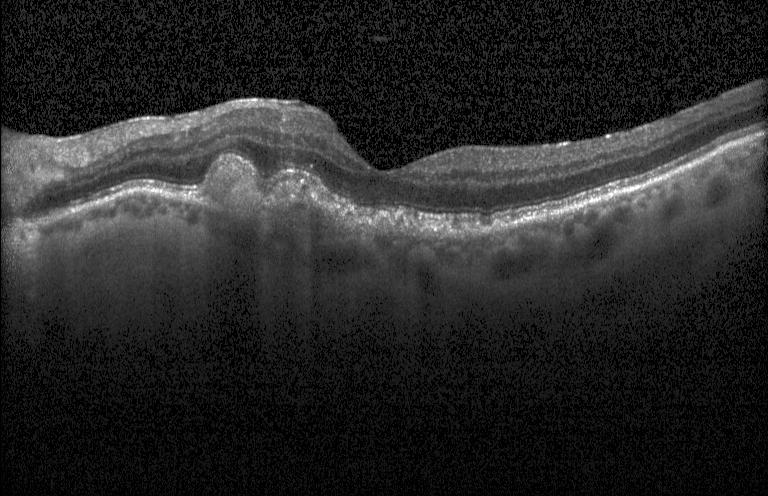

Retinal OCT cross-section showing choroidal neovascularization.